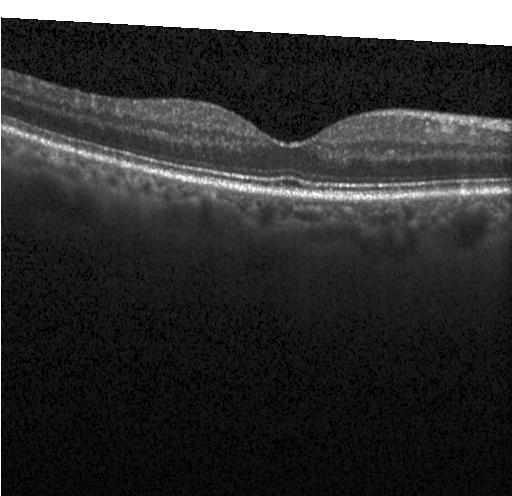 Retinal OCT cross-section. Impression: no evidence of choroidal neovascularization, diabetic macular edema, or drusen.